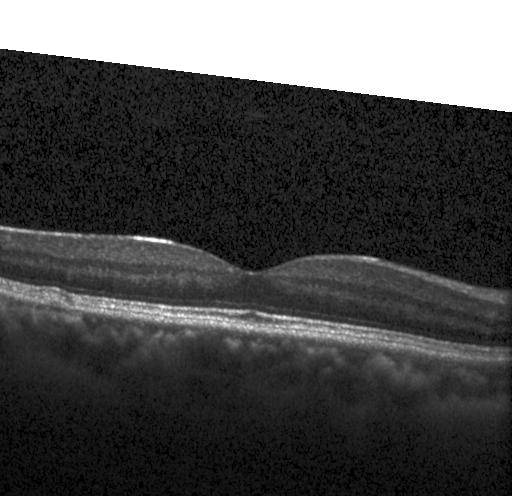
Instrument: Heidelberg Spectralis; SD-OCT; retinal OCT cross-section; centered on the fovea. Dx: neither choroidal neovascularization, diabetic macular edema, nor drusen.